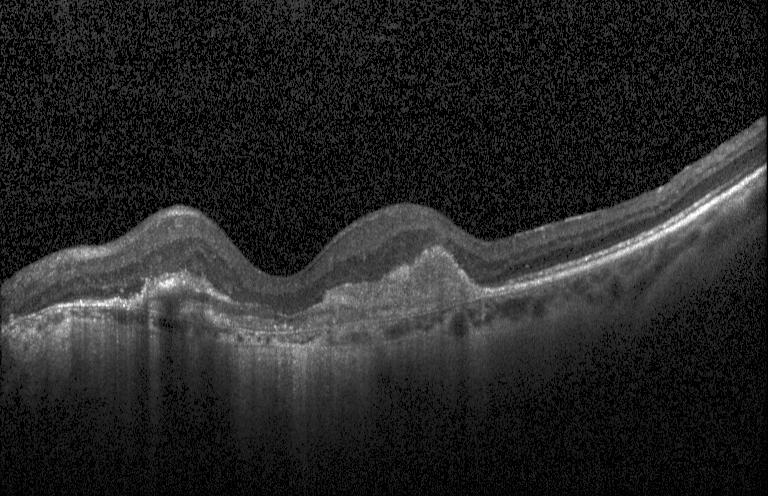 Optical coherence tomography B-scan, Heidelberg Spectralis OCT system, spectral-domain OCT. Assessment: a choroidal neovascular membrane.